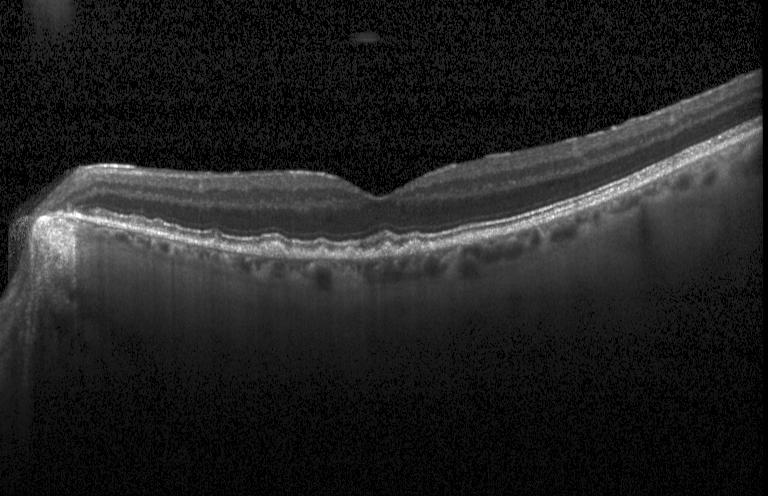
Spectral-domain OCT. OCT B-scan. Macular OCT: multiple drusen.